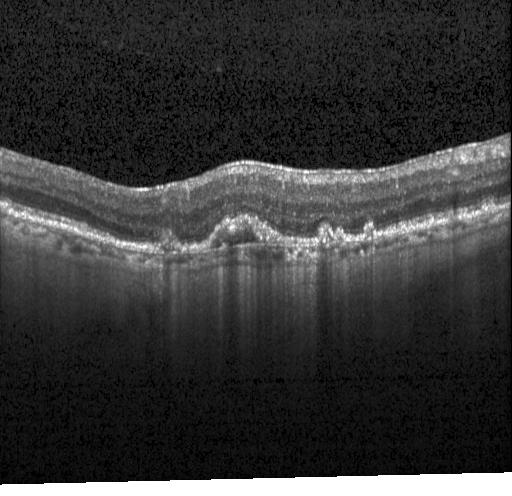

Acquired on a Heidelberg Spectralis, OCT line scan, spectral-domain optical coherence tomography, macular scan. Assessment: a choroidal neovascular membrane.